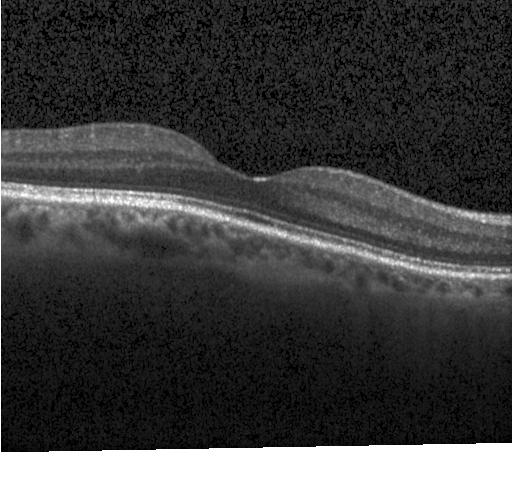

Retinal OCT cross-section. No choroidal neovascularization, no diabetic macular edema, and no drusen.